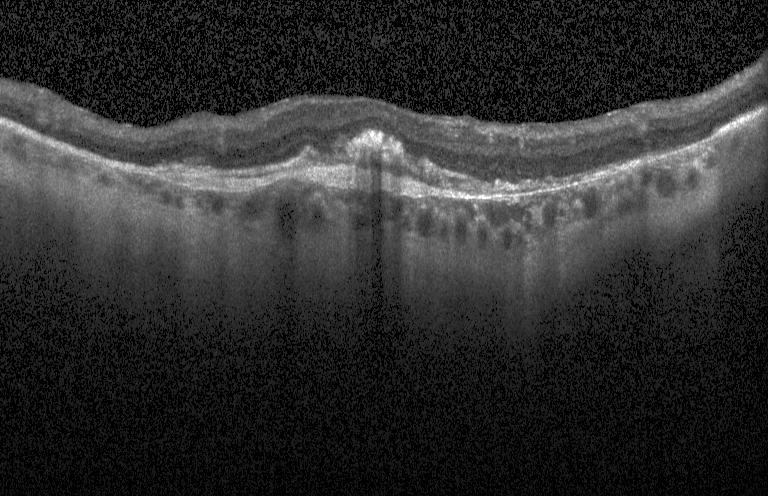

The scan shows a choroidal neovascular membrane.